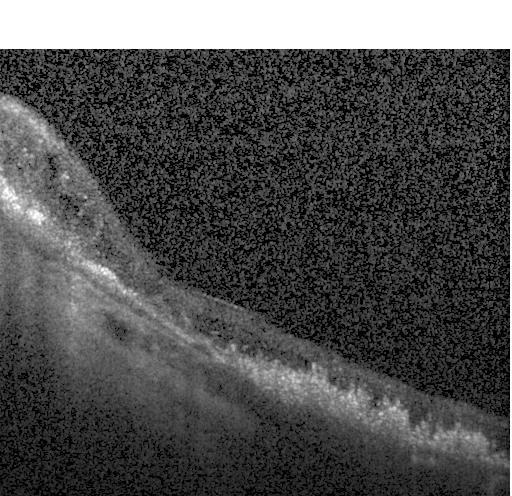

Diagnosis: a choroidal neovascular membrane.